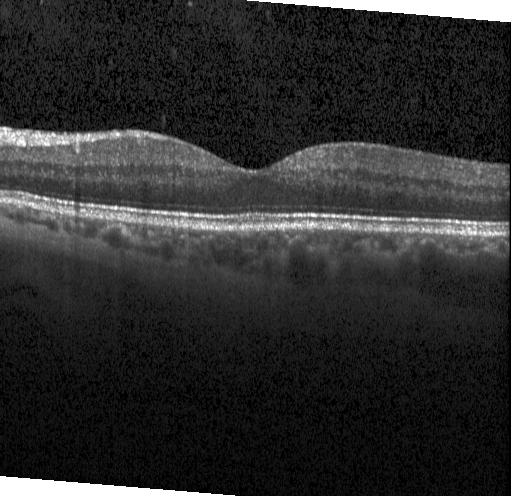

Spectral-domain optical coherence tomography. Instrument: Heidelberg Spectralis. Retinal OCT cross-section. Macular scan
The scan shows no choroidal neovascularization, diabetic macular edema, or drusen.